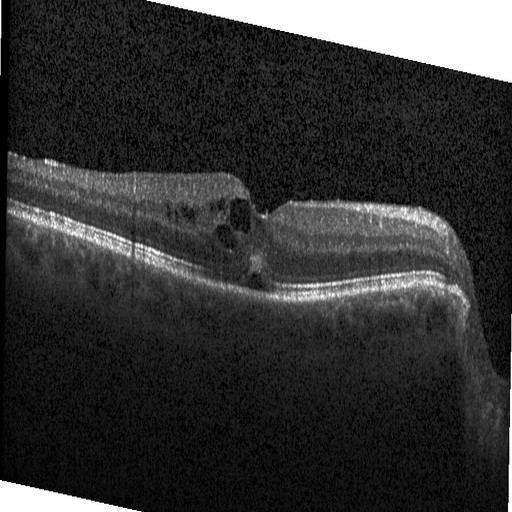
OCT finding: diabetic macular edema (DME).